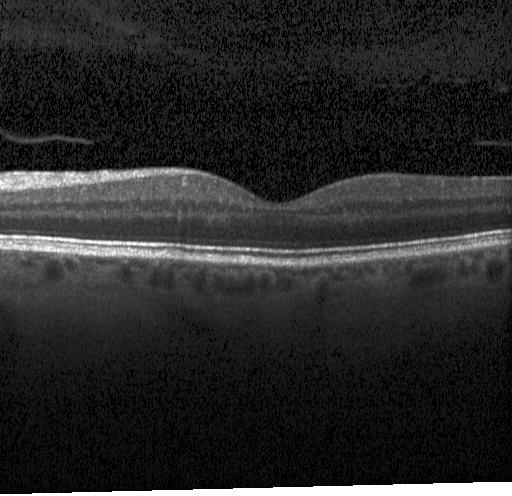
Finding: no evidence of choroidal neovascularization, diabetic macular edema, or drusen.